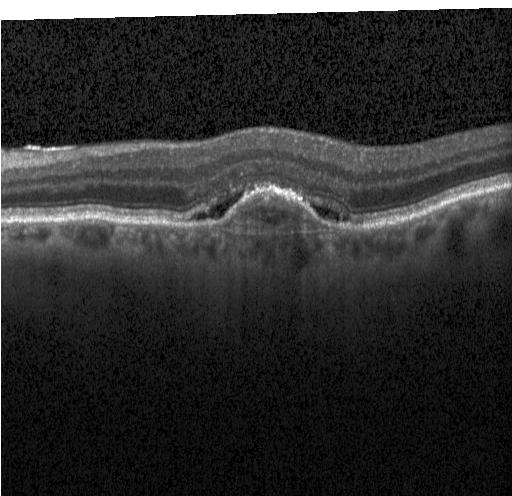
Spectral-domain optical coherence tomography, fovea-centered, retinal OCT B-scan.
Impression: choroidal neovascularization (CNV).